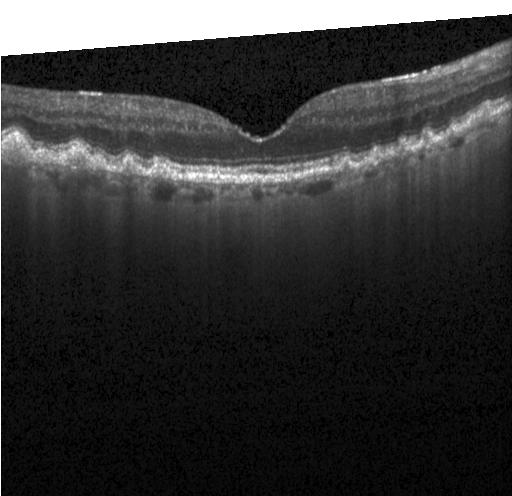
OCT B-scan showing sub-RPE drusenoid deposits.